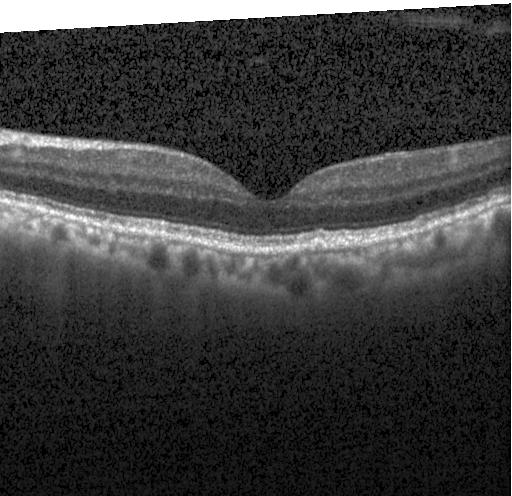

Centered on the fovea; optical coherence tomography scan — The scan shows multiple drusen.